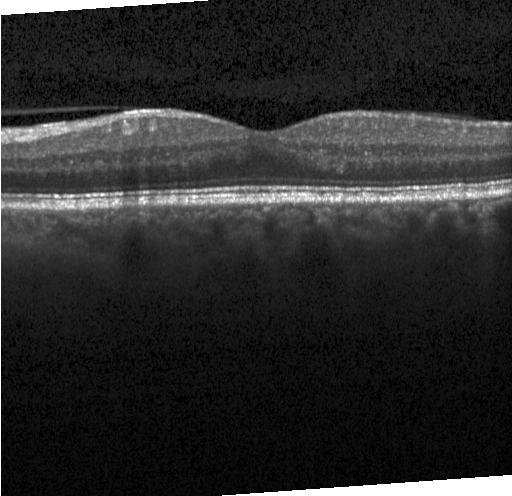

Optical coherence tomography scan; spectral-domain OCT.
Neither choroidal neovascularization, diabetic macular edema, nor drusen.